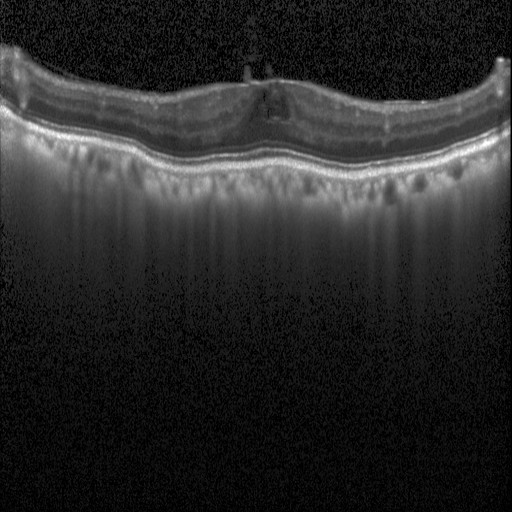
Spectral-domain OCT. Heidelberg Spectralis OCT system. Fovea-centered. Retinal OCT B-scan.
Diagnosis: diabetic macular edema.